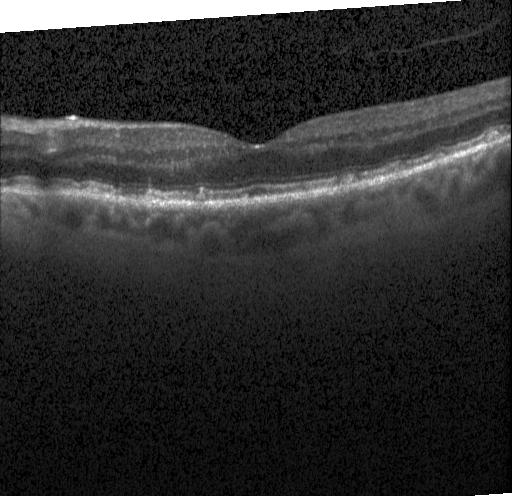
Spectral-domain OCT B-scan: sub-RPE drusenoid deposits.